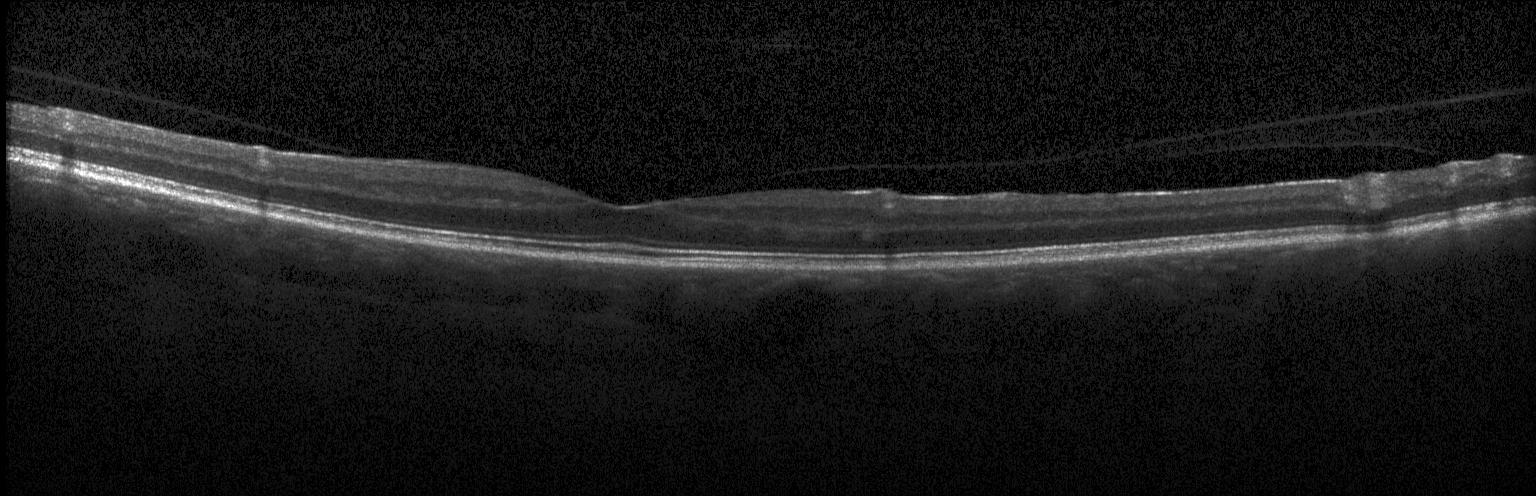 SD-OCT · retinal OCT cross-section — Finding: no evidence of choroidal neovascularization, diabetic macular edema, or drusen.